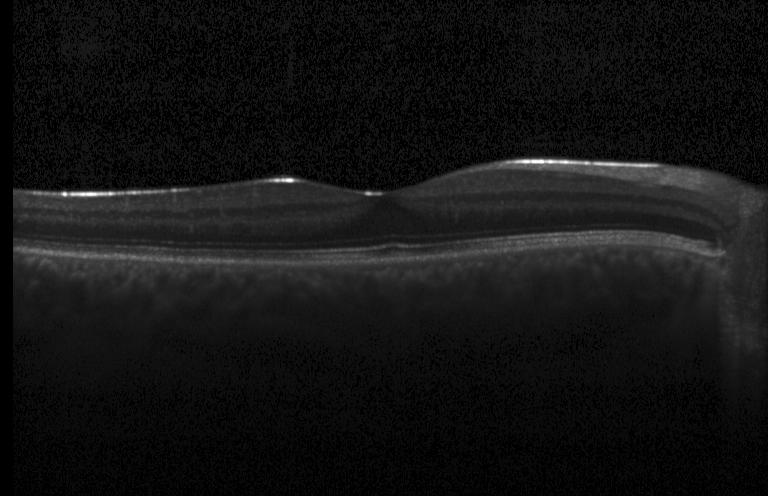

Heidelberg Spectralis · through the macula · retinal OCT cross-section — Impression: neither choroidal neovascularization, diabetic macular edema, nor drusen.